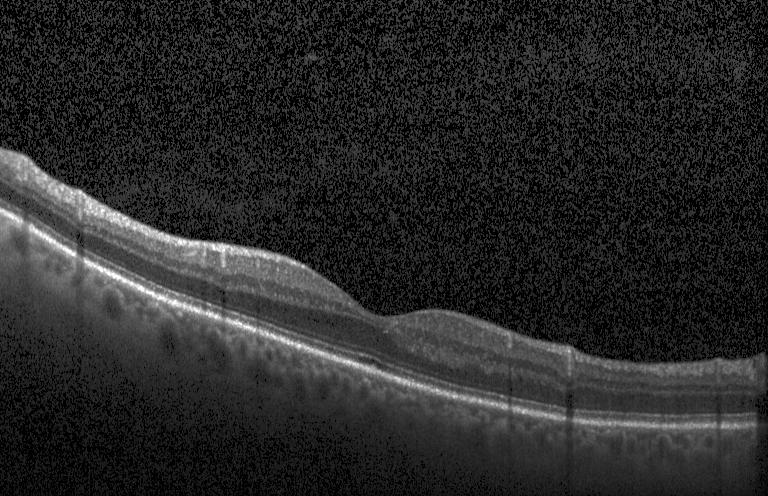

OCT line scan, horizontal scan through the fovea, Heidelberg Spectralis. The scan shows no choroidal neovascularization, diabetic macular edema, or drusen.